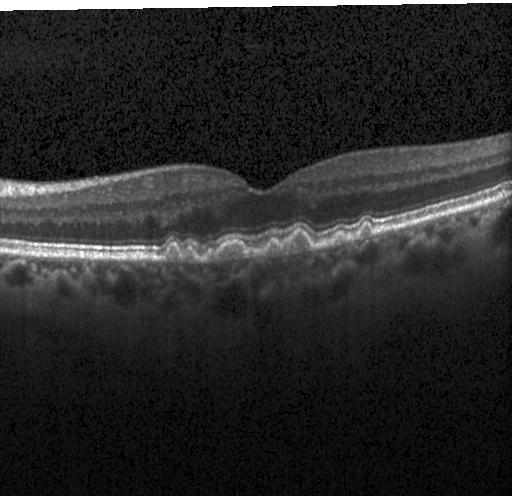 OCT line scan; SD-OCT
Finding: multiple drusen.